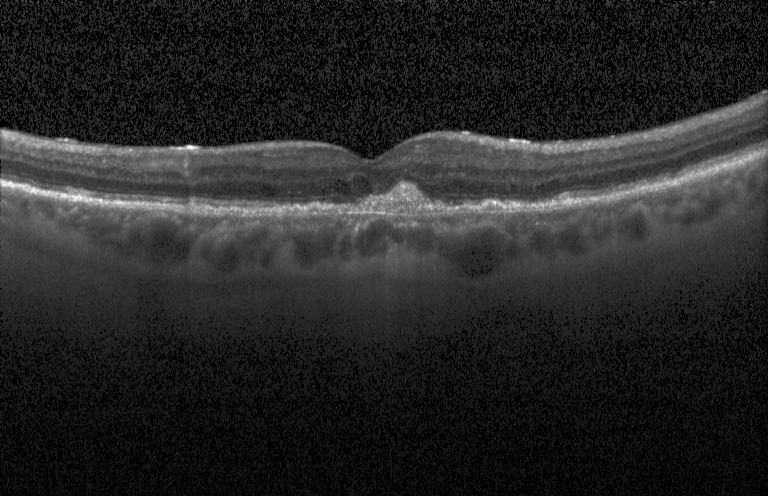 OCT line scan.
Impression: a choroidal neovascular membrane.